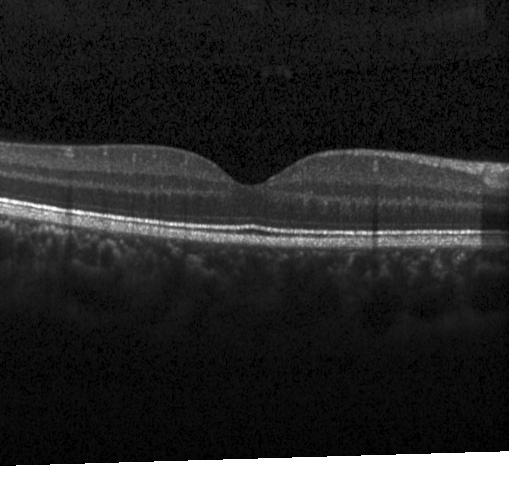 Optical coherence tomography B-scan.
Impression: no CNV, DME, or drusen.